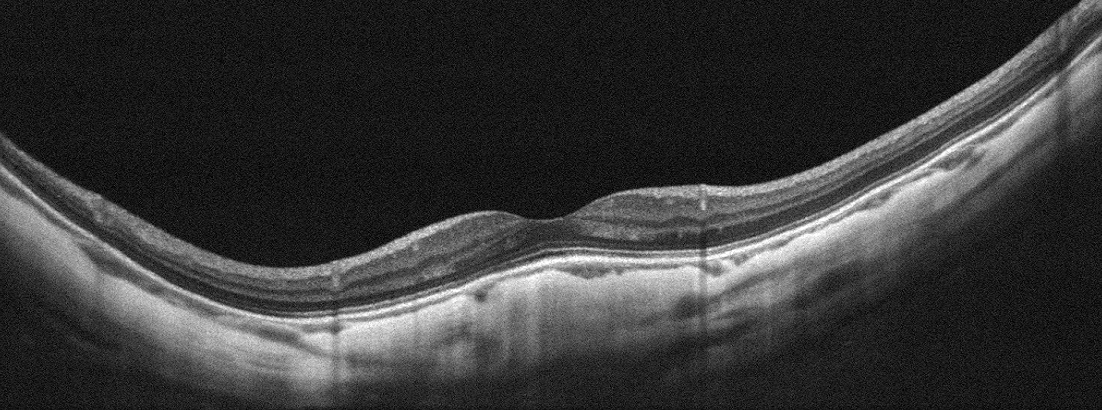

Fovea-centered; instrument: Optovue Avanti RTVue XR; retinal OCT B-scan.
This B-scan demonstrates absence of AMD, DME, ERM, RAO, RVO, and vitreomacular interface disease.